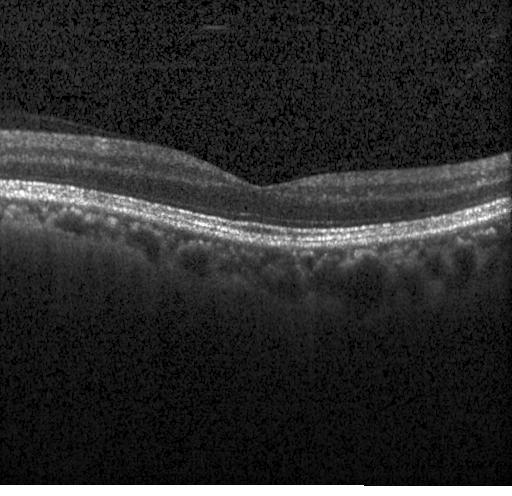

Retinal OCT B-scan. Acquired on a Heidelberg Spectralis
Impression: no evidence of CNV, DME, or drusen.